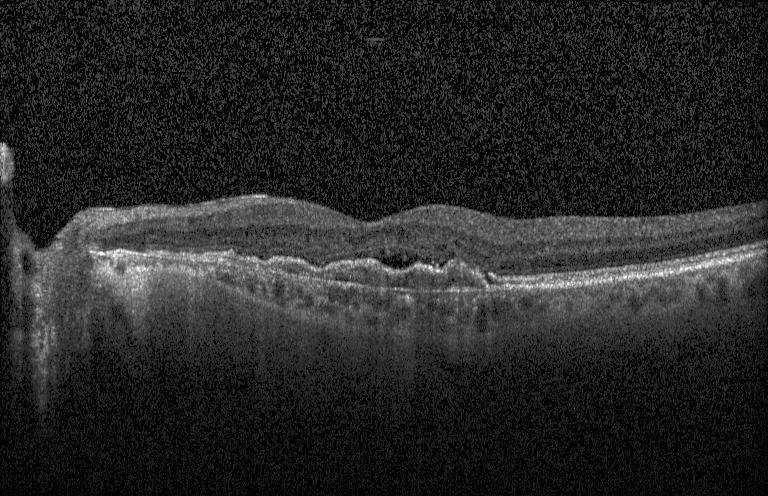

Centered on the fovea. Acquired on a Heidelberg Spectralis. SD-OCT. Retinal OCT cross-section. OCT finding: CNV.